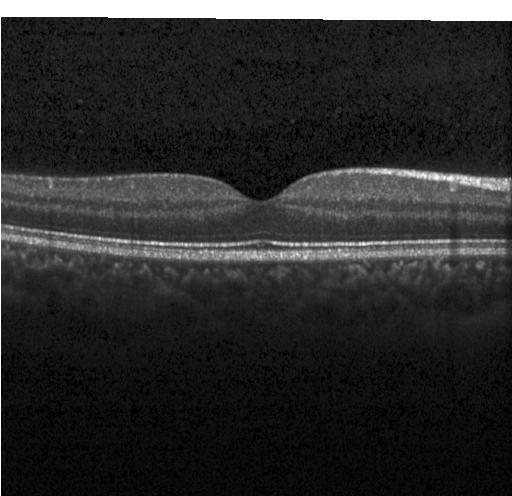

Retinal OCT cross-section — Finding: no choroidal neovascularization, diabetic macular edema, or drusen.